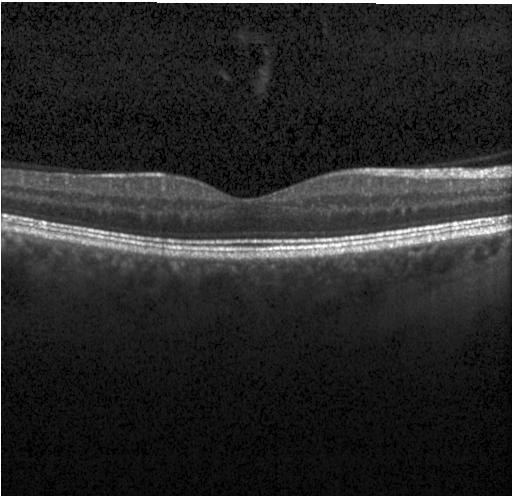

Spectral-domain optical coherence tomography · retinal OCT cross-section · instrument: Heidelberg Spectralis · horizontal scan through the fovea
Assessment: no choroidal neovascularization, no diabetic macular edema, and no drusen.